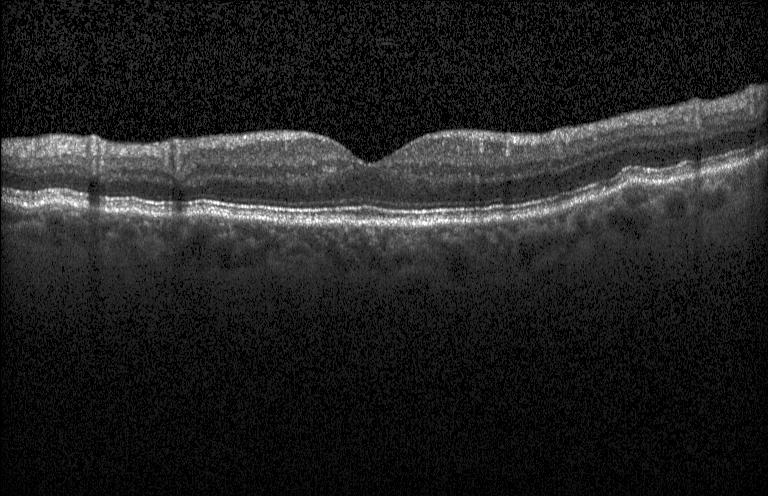 OCT finding: sub-RPE drusenoid deposits.